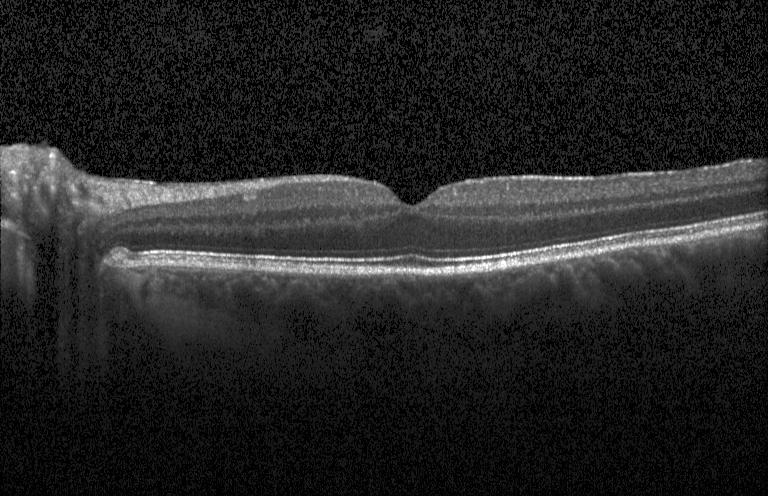 OCT finding: no choroidal neovascularization, no diabetic macular edema, and no drusen.